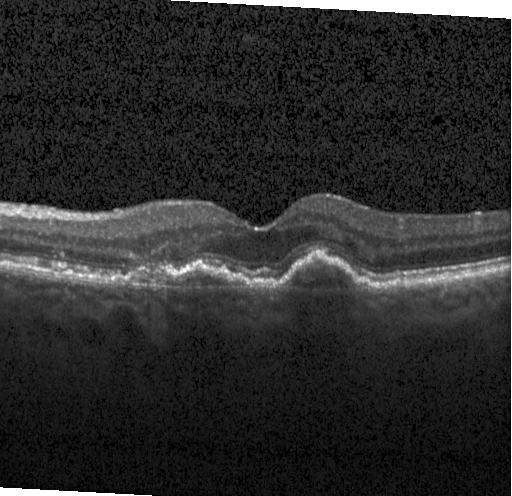 Spectral-domain OCT; retinal OCT cross-section — Finding: a choroidal neovascular membrane.